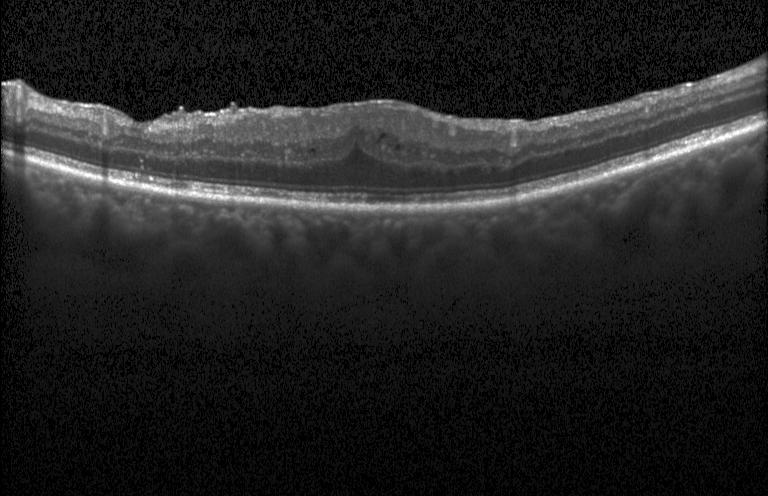 Macular OCT: neither CNV, DME, nor drusen.